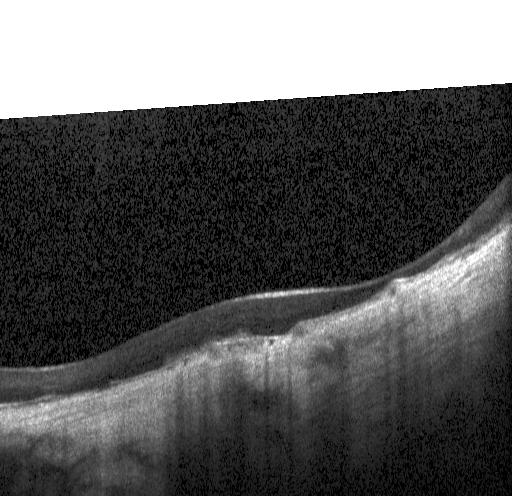
This B-scan demonstrates a choroidal neovascular membrane.